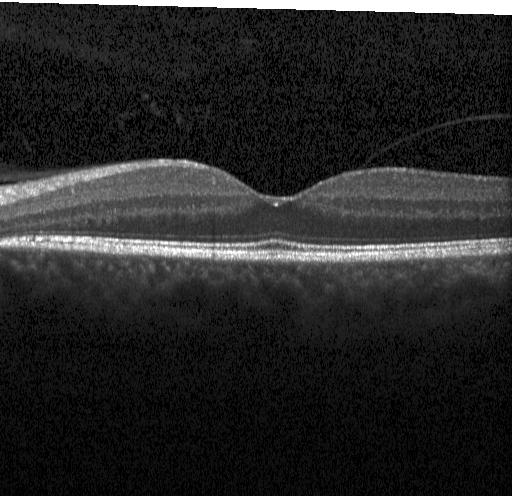

OCT B-scan — Impression: no choroidal neovascularization, no diabetic macular edema, and no drusen.